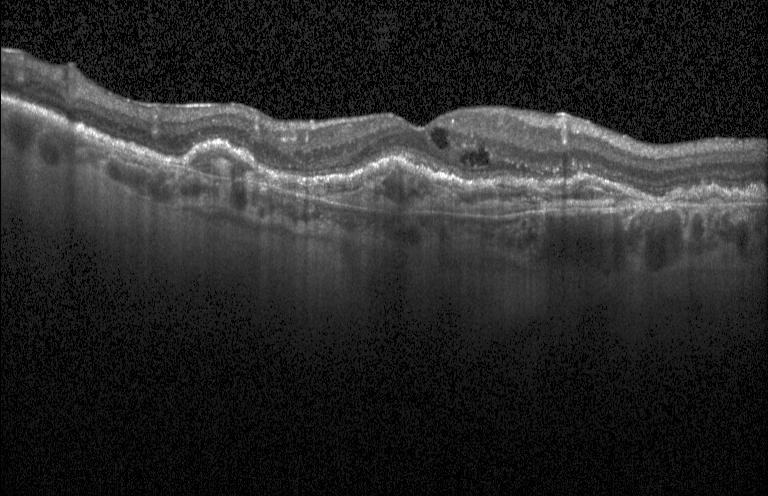 Macular OCT demonstrating a choroidal neovascular membrane.